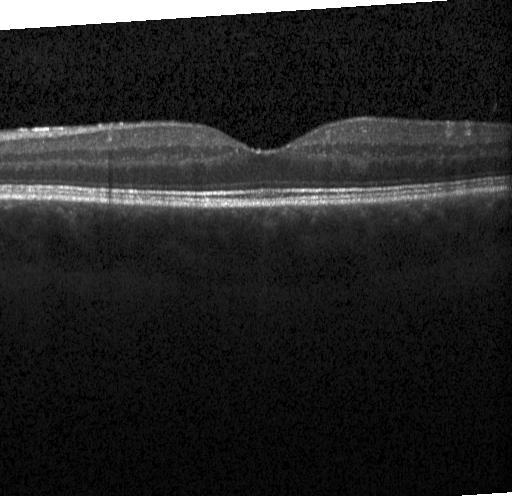

Spectral-domain OCT · instrument: Heidelberg Spectralis · through the macula · optical coherence tomography B-scan — Finding: no CNV, no DME, and no drusen.